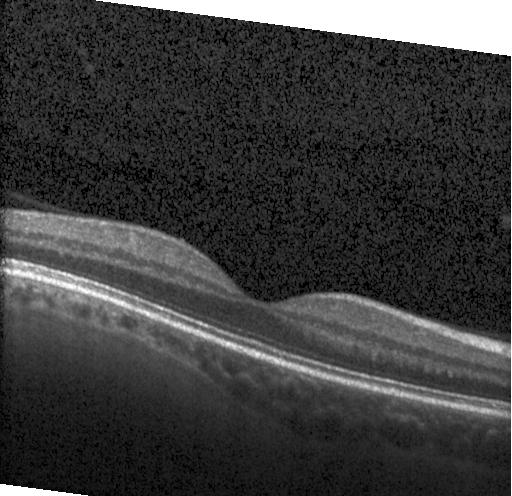 Macular OCT: neither choroidal neovascularization, diabetic macular edema, nor drusen.